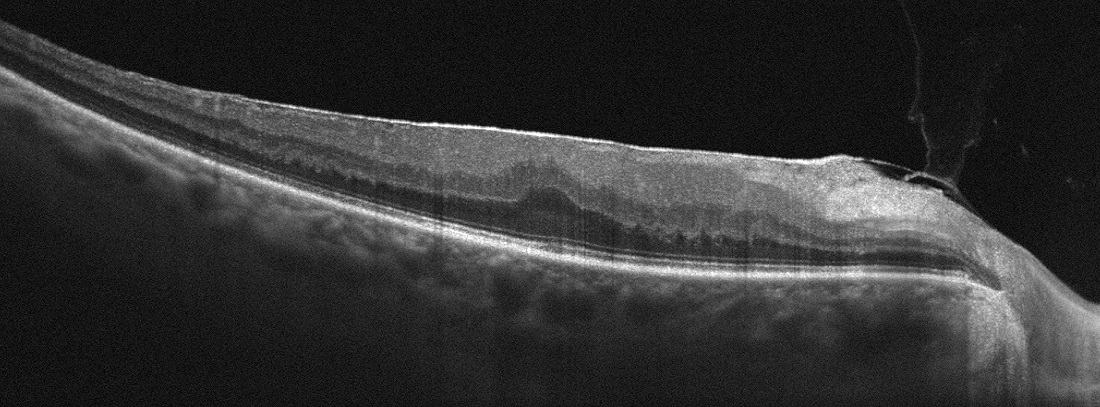 Macular OCT: epiretinal membrane (ERM).